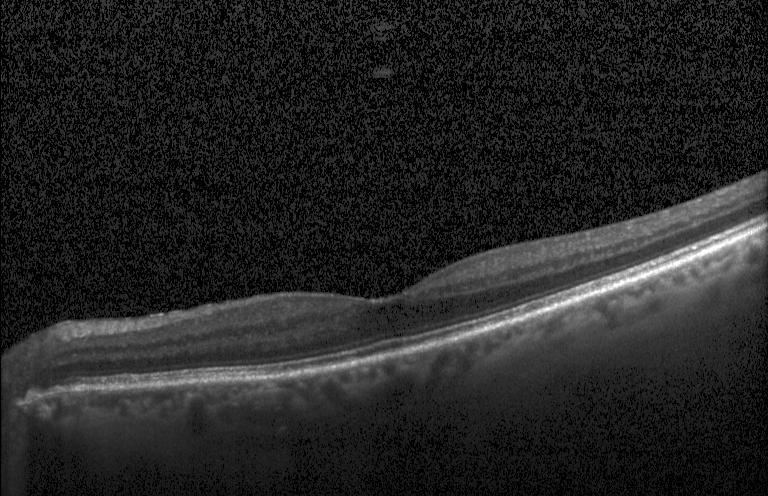

Retinal OCT B-scan. Finding: no evidence of CNV, DME, or drusen.